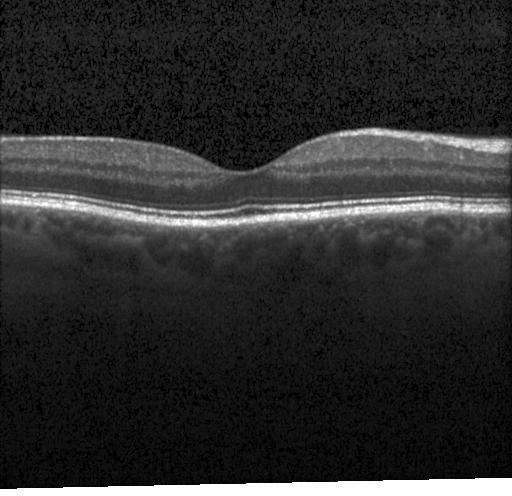 Retinal OCT cross-section showing no choroidal neovascularization, no diabetic macular edema, and no drusen.